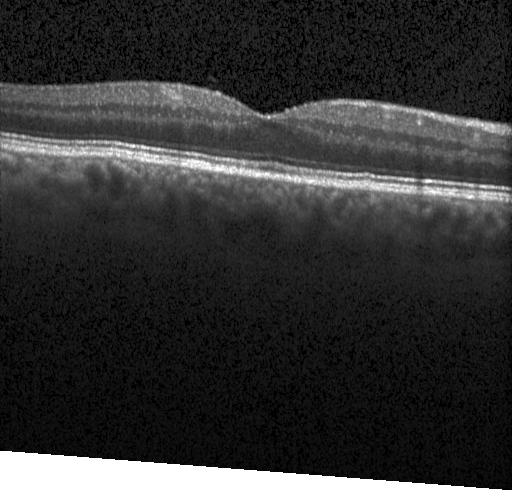 Heidelberg Spectralis, optical coherence tomography scan, SD-OCT, centered on the fovea — Assessment: no evidence of choroidal neovascularization, diabetic macular edema, or drusen.